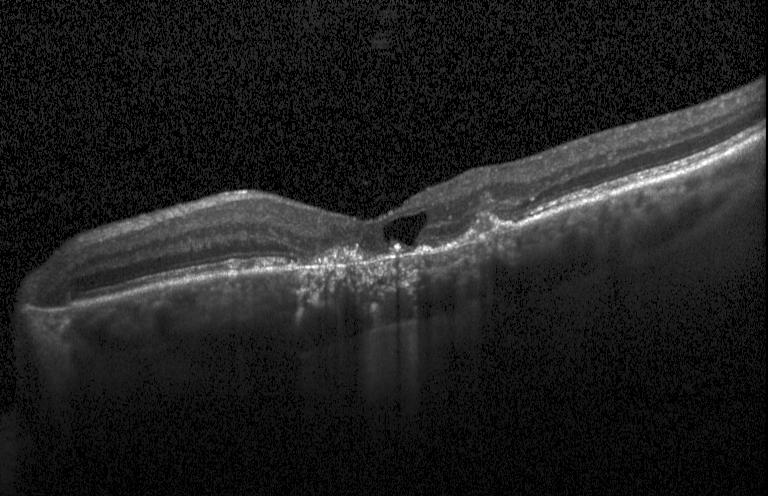

OCT line scan — Finding: a choroidal neovascular membrane.